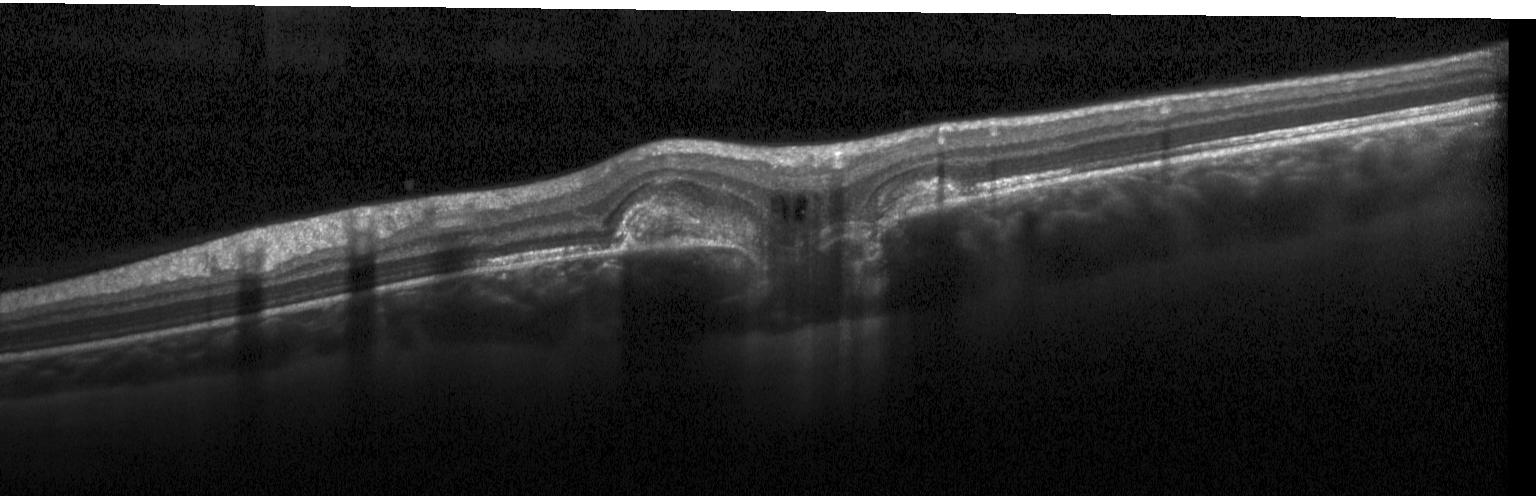

OCT line scan. Dx: choroidal neovascularization (CNV).